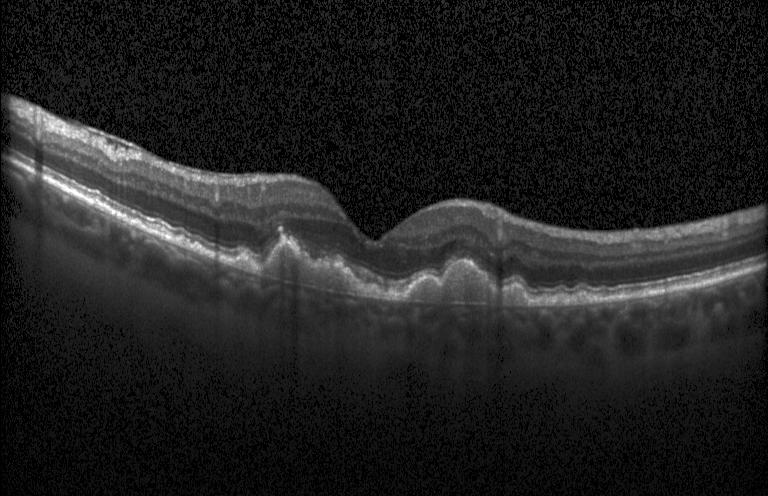
Macular OCT demonstrating drusen.